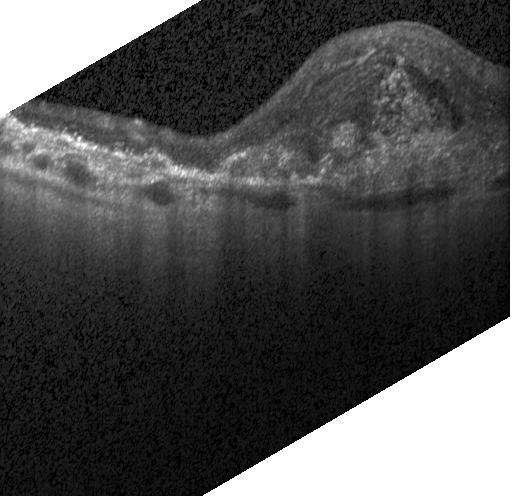
Spectral-domain OCT B-scan: a choroidal neovascular membrane.